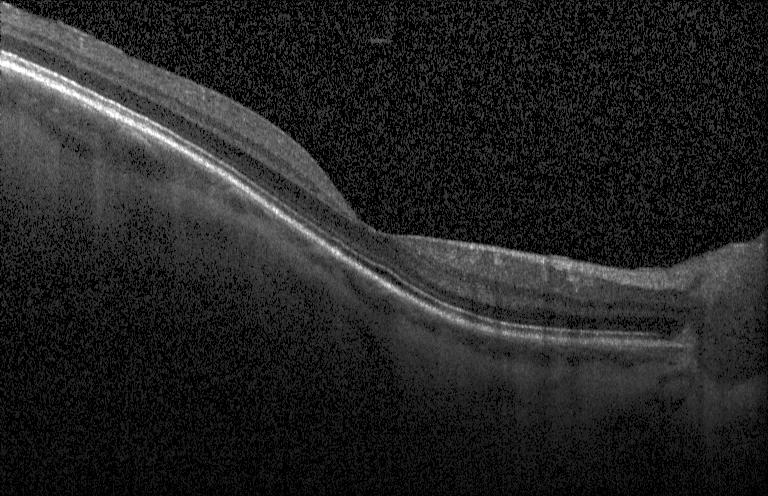

Spectral-domain optical coherence tomography; retinal OCT B-scan; macular scan; instrument: Heidelberg Spectralis.
Impression: no choroidal neovascularization, diabetic macular edema, or drusen.